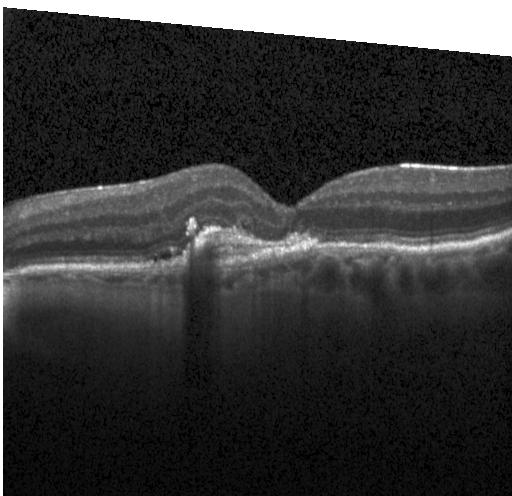
OCT line scan; SD-OCT
Impression: a choroidal neovascular membrane.